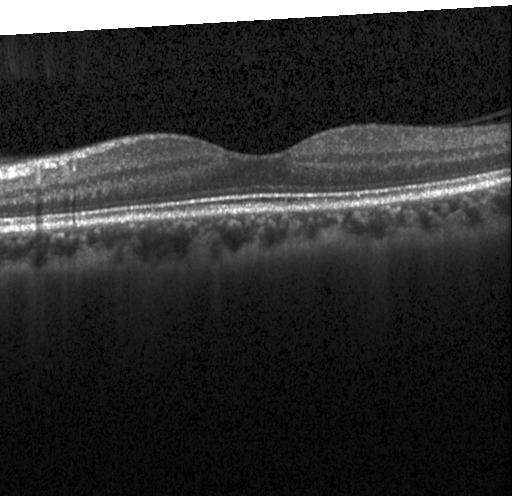 Finding: no evidence of choroidal neovascularization, diabetic macular edema, or drusen.